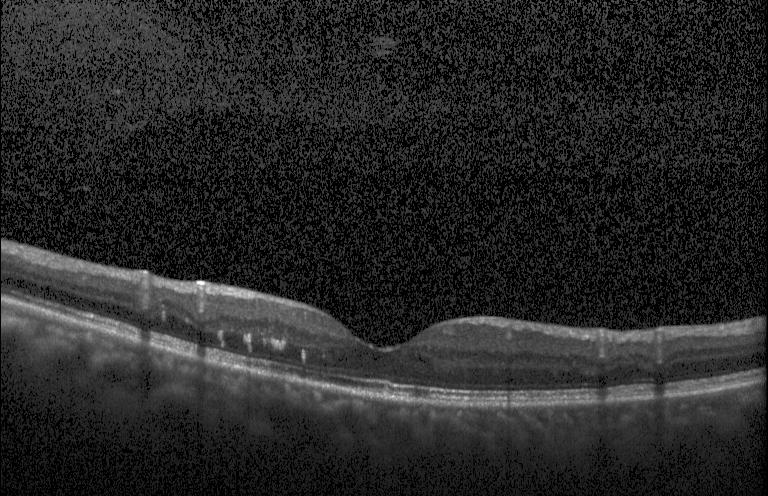

Acquired on a Heidelberg Spectralis; optical coherence tomography scan — This B-scan demonstrates neither choroidal neovascularization, diabetic macular edema, nor drusen.